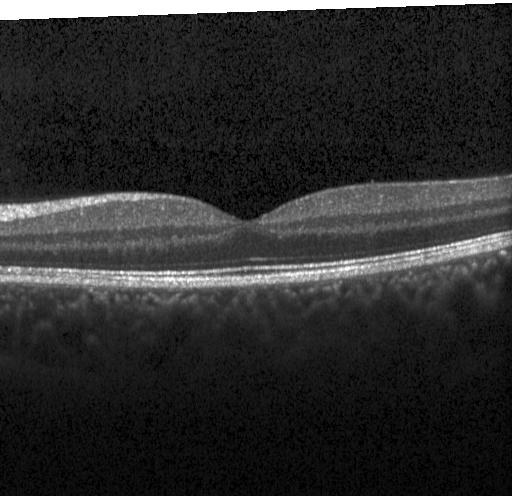 Retinal OCT cross-section, spectral-domain OCT. Macular OCT: no CNV, DME, or drusen.